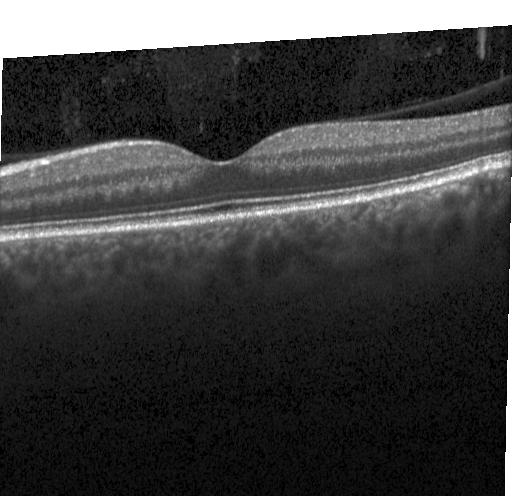
Impression: no evidence of choroidal neovascularization, diabetic macular edema, or drusen.